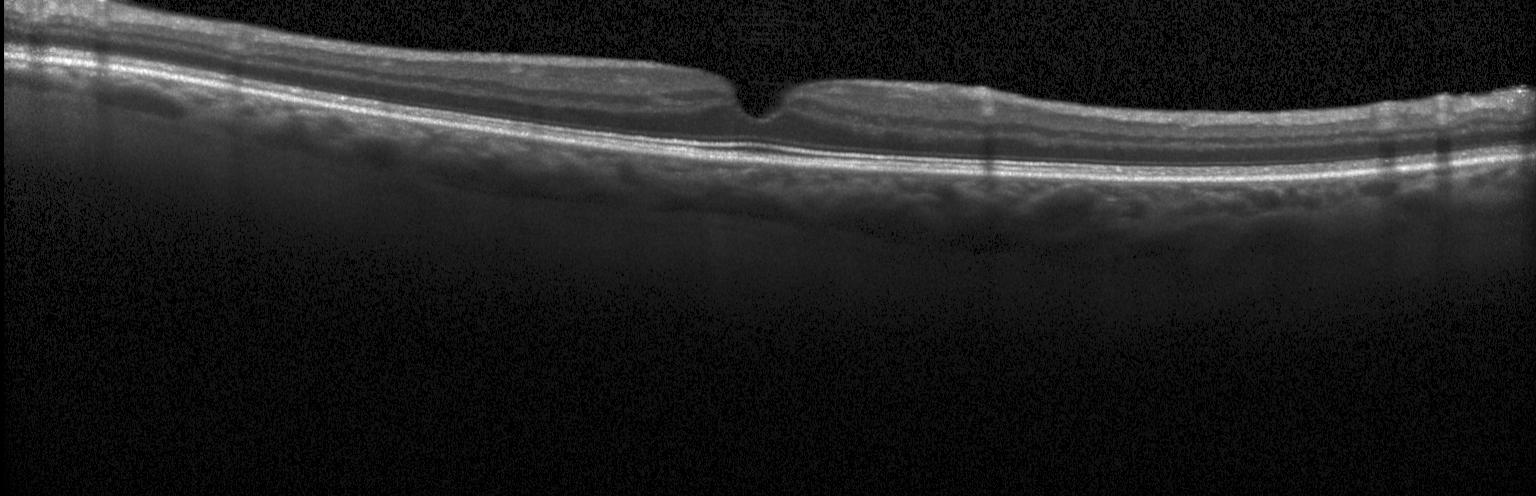 Impression: no CNV, no DME, and no drusen.